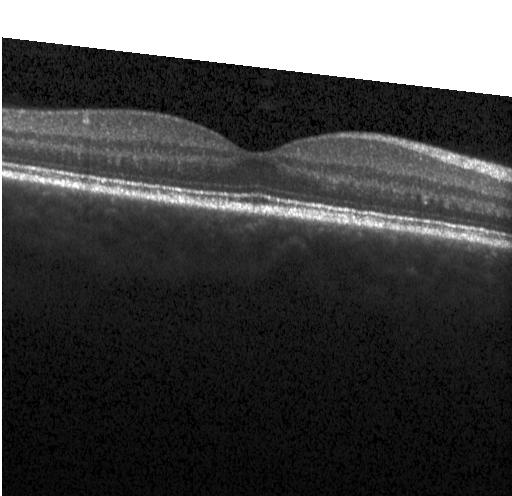 Spectral-domain optical coherence tomography, optical coherence tomography scan — Impression: no CNV, DME, or drusen.